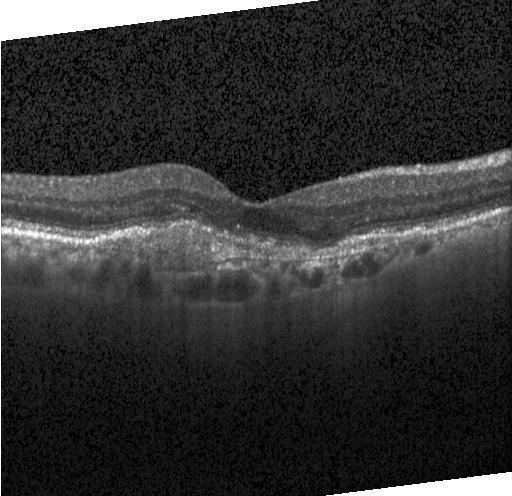 Retinal OCT cross-section; spectral-domain optical coherence tomography
Finding: CNV.